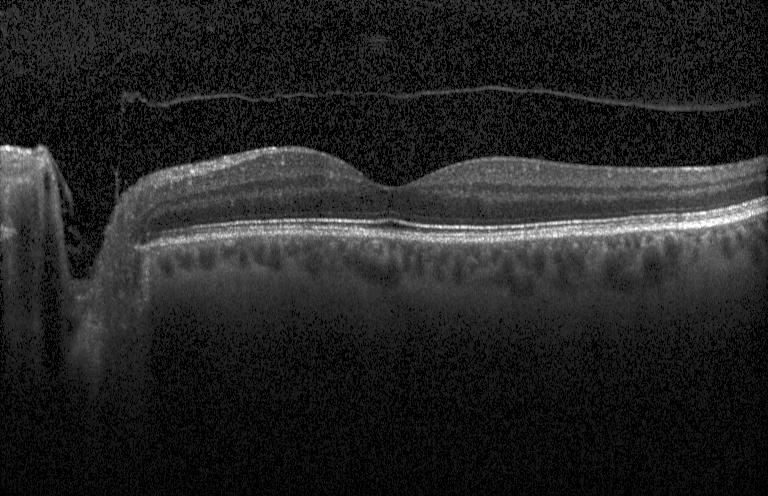 Heidelberg Spectralis; optical coherence tomography B-scan; horizontal scan through the fovea; spectral-domain OCT
Finding: neither choroidal neovascularization, diabetic macular edema, nor drusen.